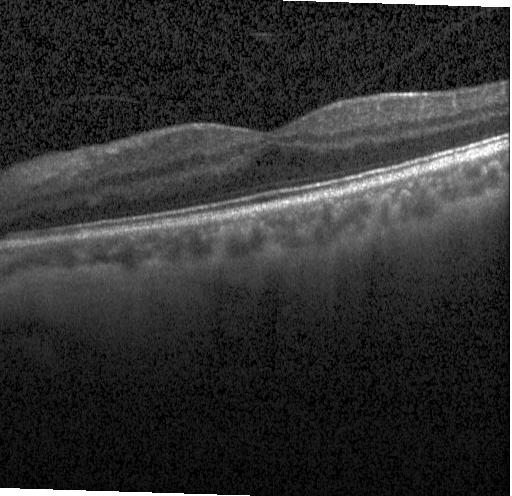 Diagnosis: neither choroidal neovascularization, diabetic macular edema, nor drusen.